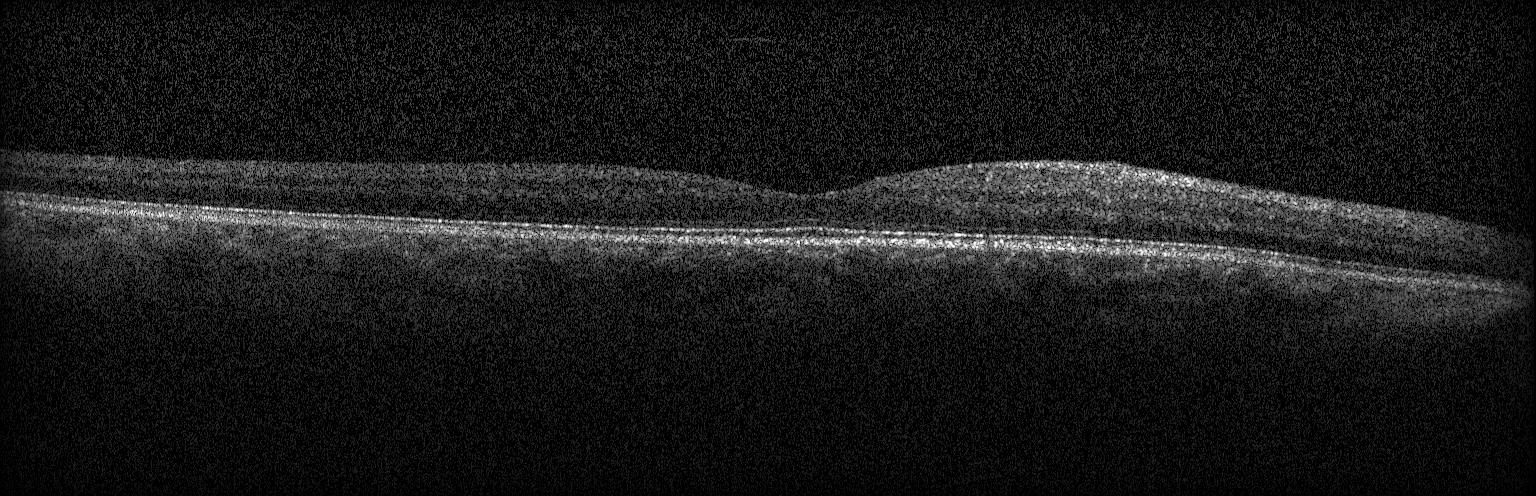
Diagnosis: no evidence of CNV, DME, or drusen.